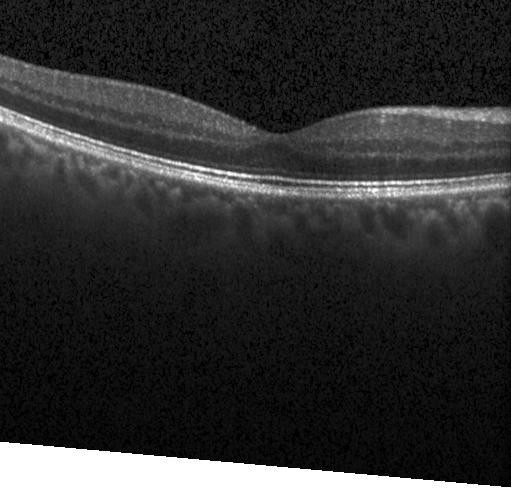 This B-scan demonstrates neither choroidal neovascularization, diabetic macular edema, nor drusen.